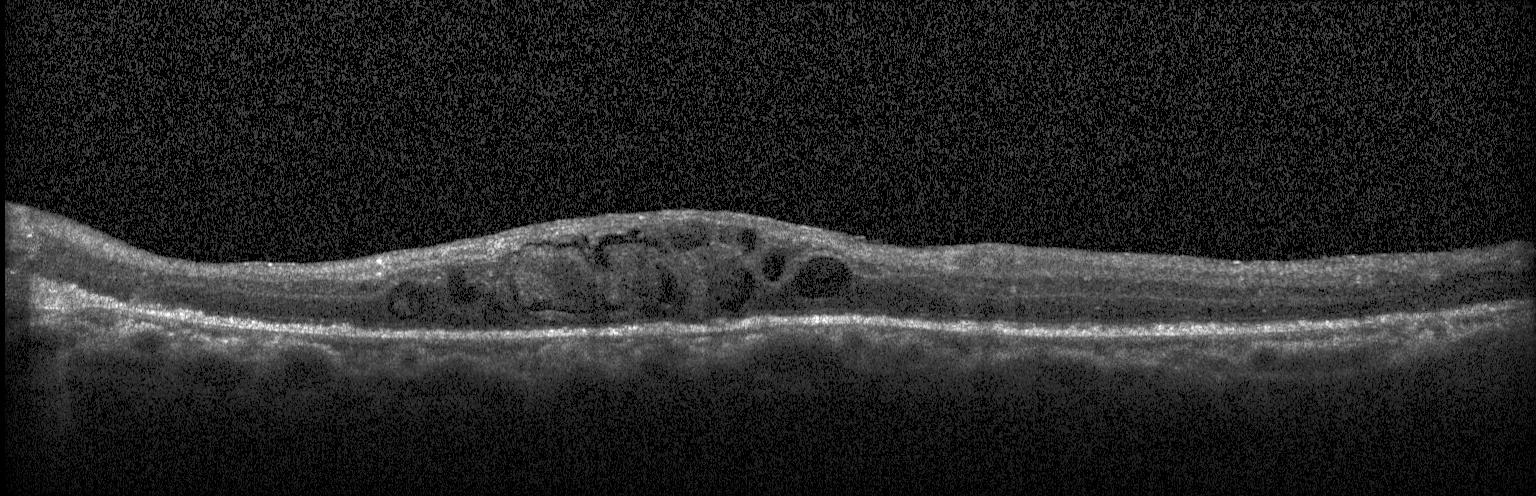

Macular scan, Heidelberg Spectralis OCT system, optical coherence tomography B-scan.
Impression: diabetic macular edema (DME).